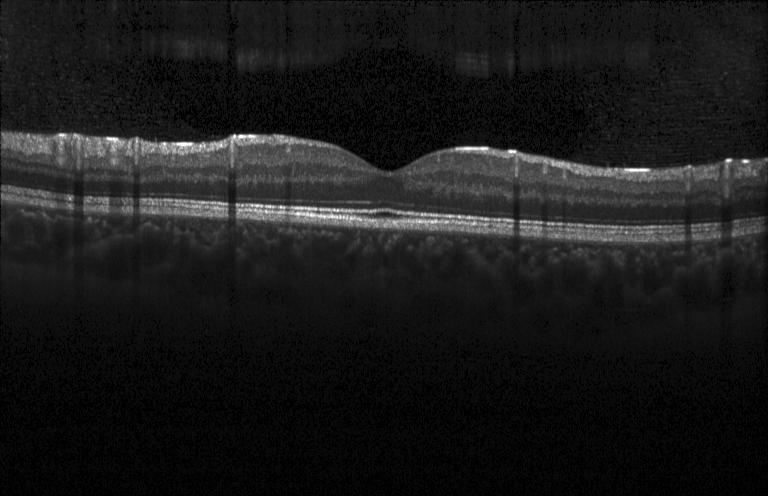
No evidence of CNV, DME, or drusen.